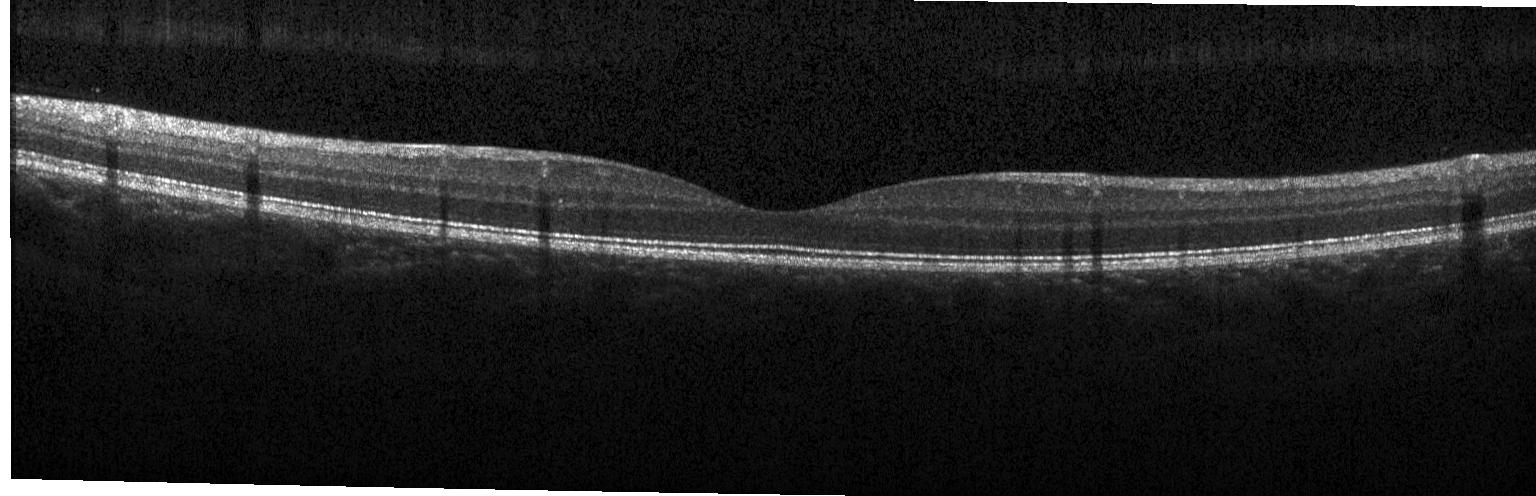
OCT finding: neither choroidal neovascularization, diabetic macular edema, nor drusen.